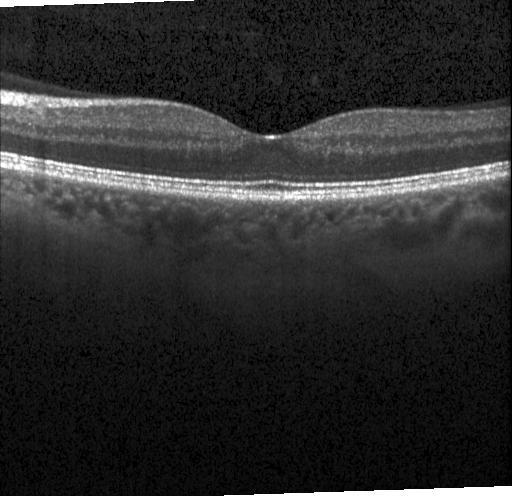
OCT B-scan — Finding: no CNV, no DME, and no drusen.